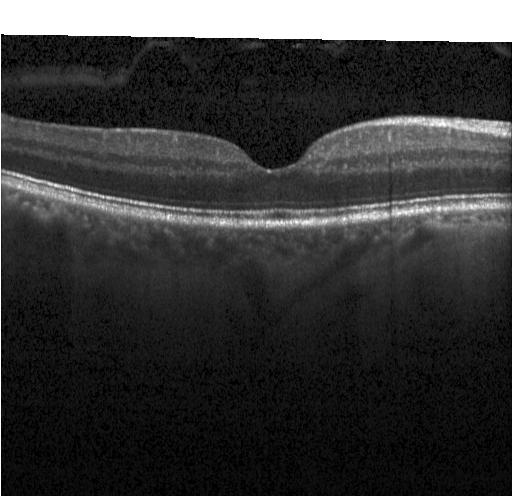 Retinal OCT cross-section. Instrument: Heidelberg Spectralis
Assessment: neither choroidal neovascularization, diabetic macular edema, nor drusen.